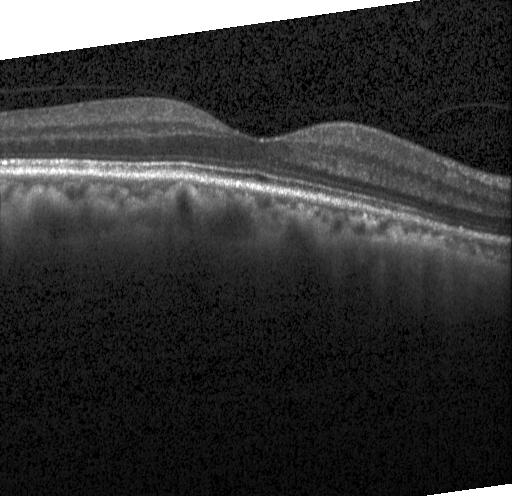 Retinal OCT B-scan
Diagnosis: neither choroidal neovascularization, diabetic macular edema, nor drusen.